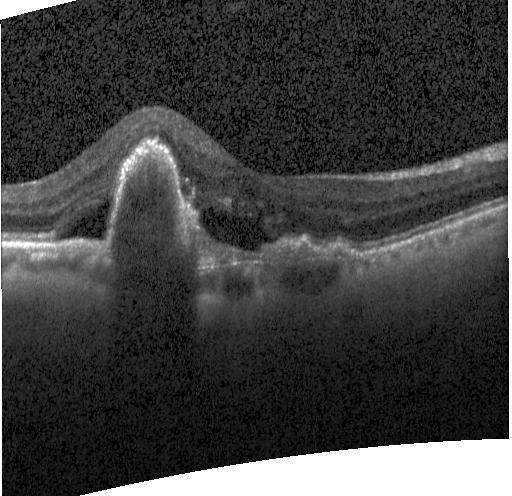

Retinal OCT cross-section, SD-OCT, Heidelberg Spectralis.
Finding: a choroidal neovascular membrane.